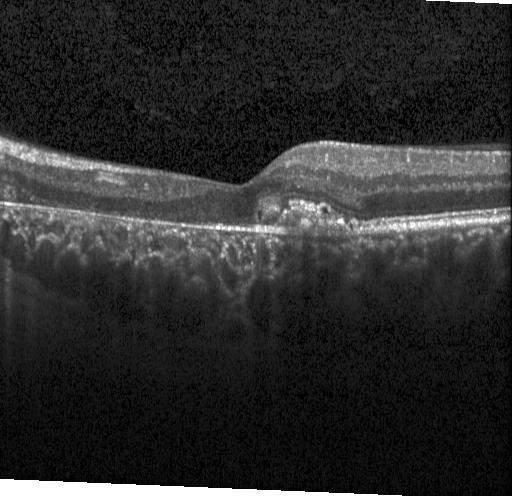

This B-scan demonstrates a choroidal neovascular membrane.